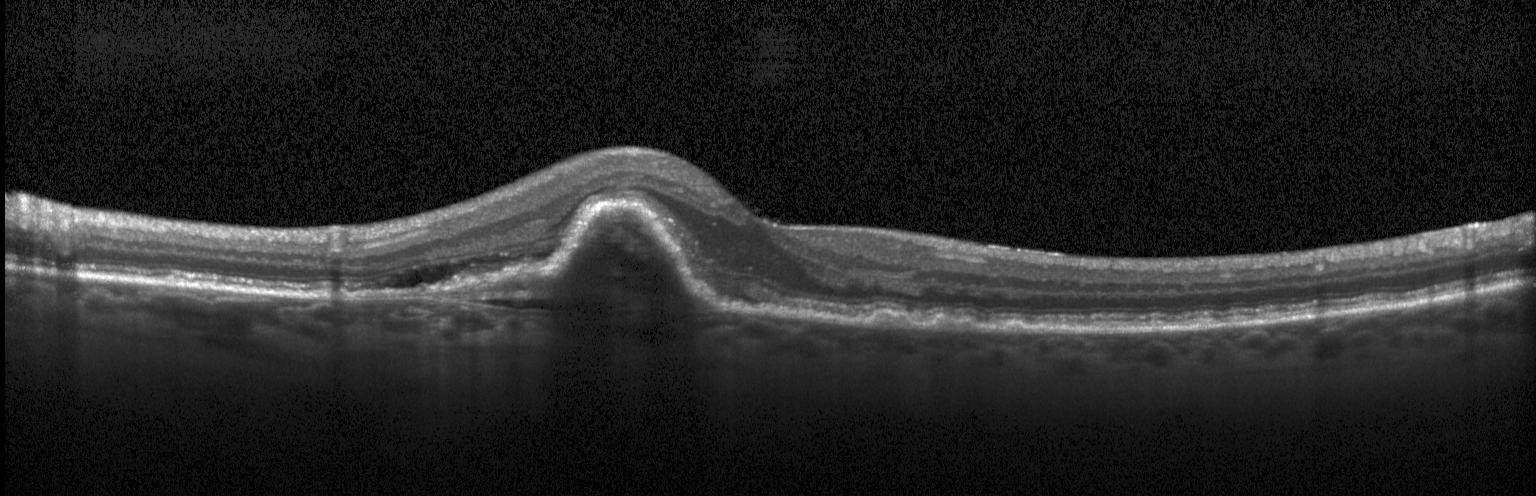 Optical coherence tomography B-scan · SD-OCT. Assessment: a choroidal neovascular membrane.